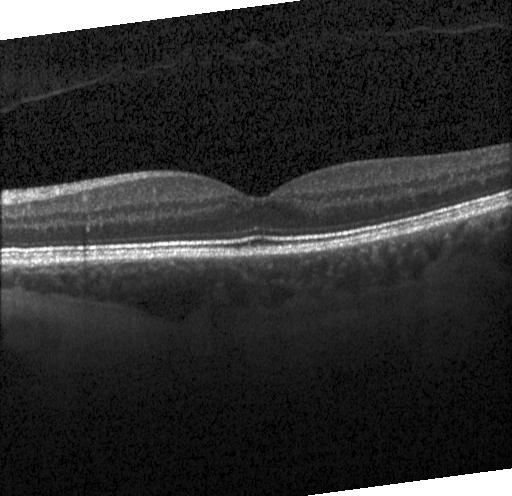 Optical coherence tomography B-scan; SD-OCT.
Impression: no choroidal neovascularization, diabetic macular edema, or drusen.